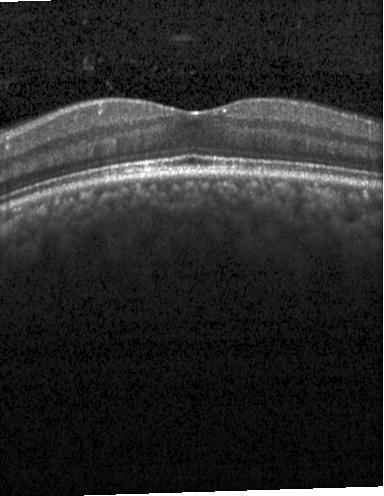 Retinal OCT B-scan; fovea-centered; SD-OCT. Macular OCT: no choroidal neovascularization, diabetic macular edema, or drusen.